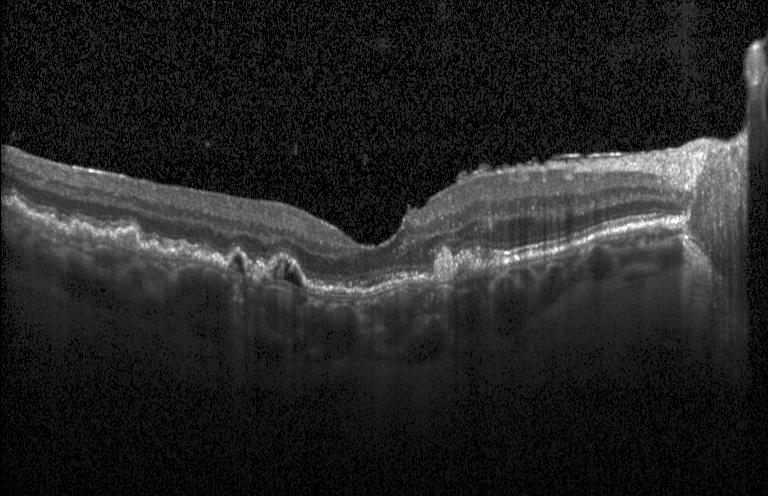 OCT B-scan; spectral-domain OCT — The scan shows a choroidal neovascular membrane.